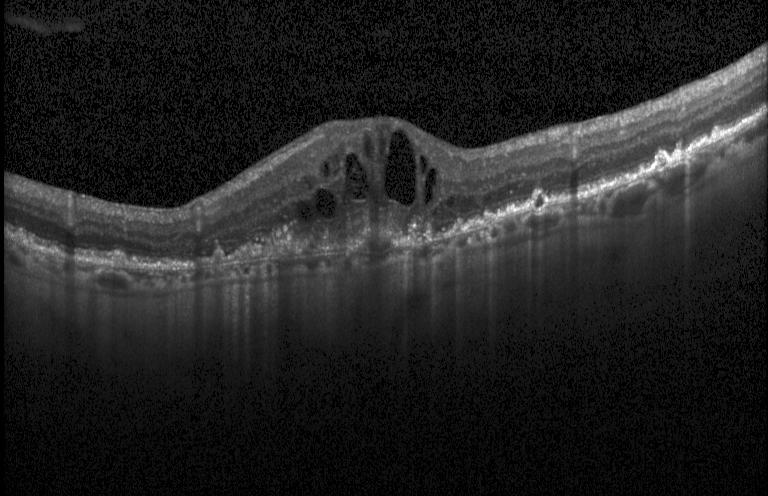

Centered on the fovea, Heidelberg Spectralis OCT system, spectral-domain OCT, OCT line scan
OCT finding: CNV.